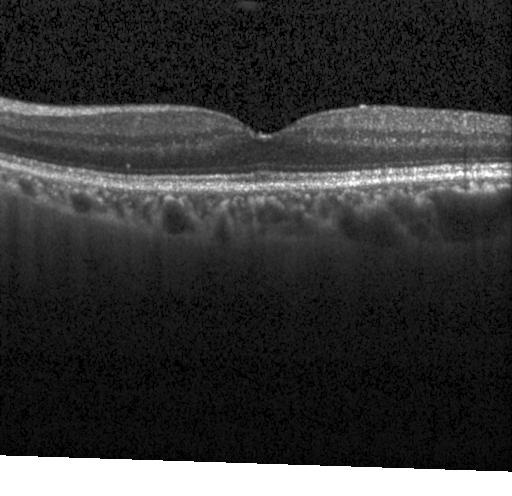
Assessment: no choroidal neovascularization, no diabetic macular edema, and no drusen.